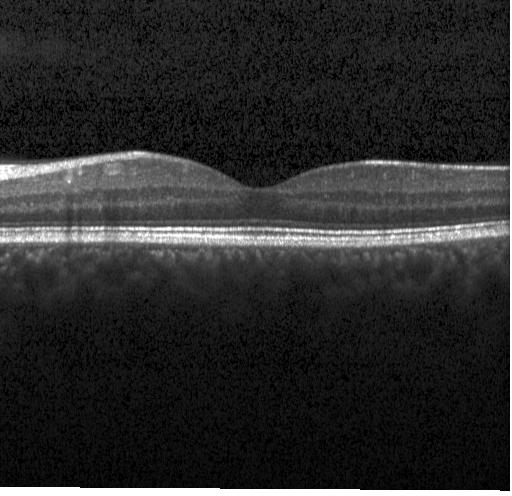 Impression: no evidence of choroidal neovascularization, diabetic macular edema, or drusen.